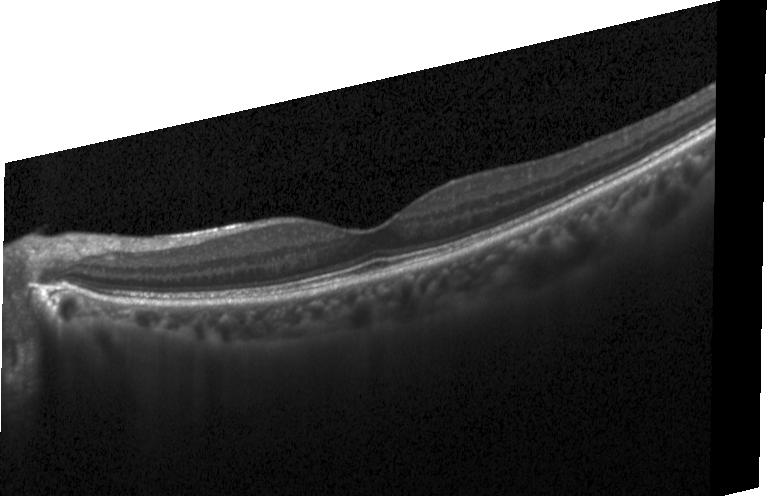 Macular OCT: no evidence of choroidal neovascularization, diabetic macular edema, or drusen.